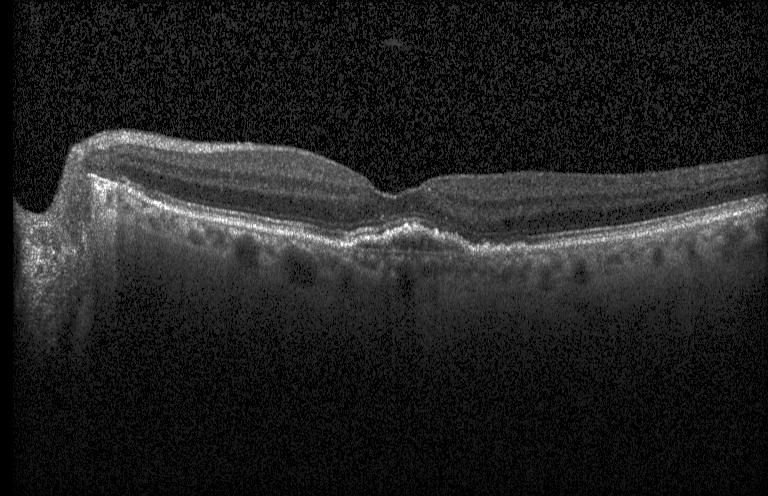
Impression: a choroidal neovascular membrane.